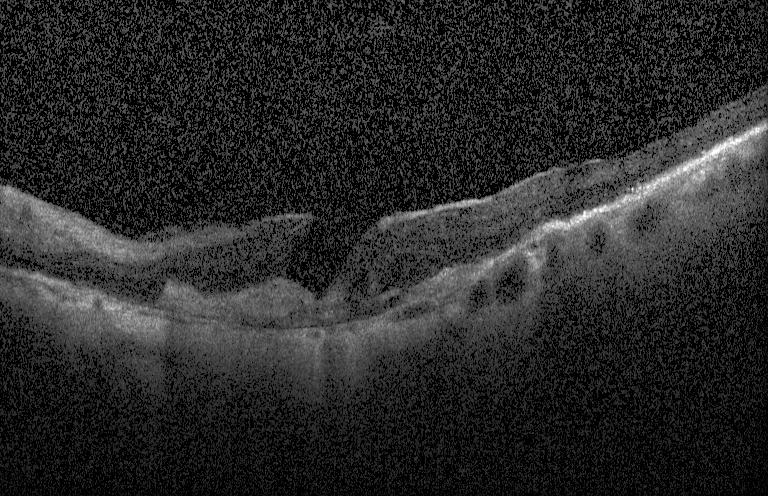
Heidelberg Spectralis. Retinal OCT cross-section. Spectral-domain OCT.
Impression: choroidal neovascularization (CNV).